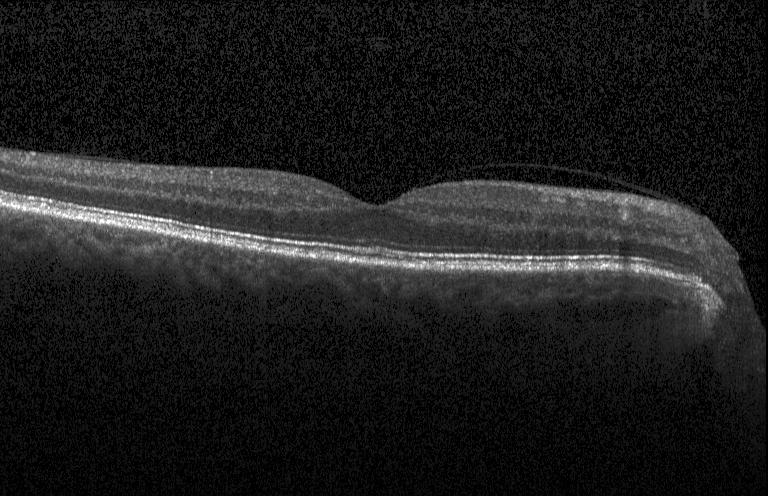
SD-OCT; macular scan; optical coherence tomography B-scan; Heidelberg Spectralis OCT system.
Diagnosis: no CNV, no DME, and no drusen.